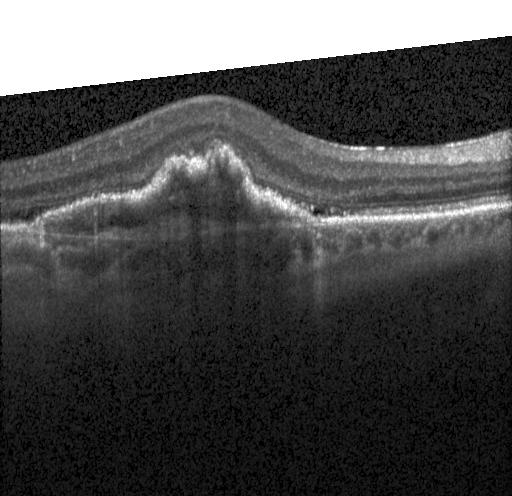

Macular OCT demonstrating choroidal neovascularization (CNV).